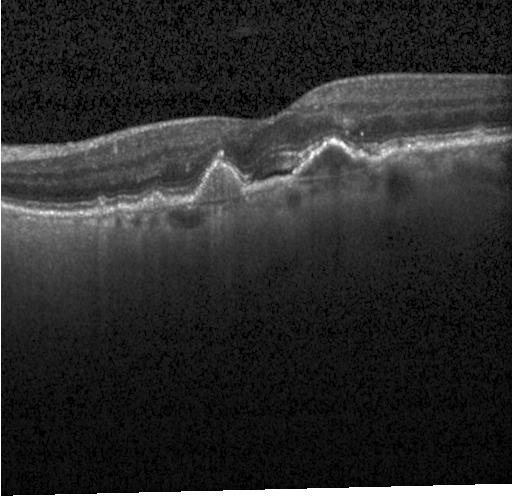
Assessment: choroidal neovascularization.